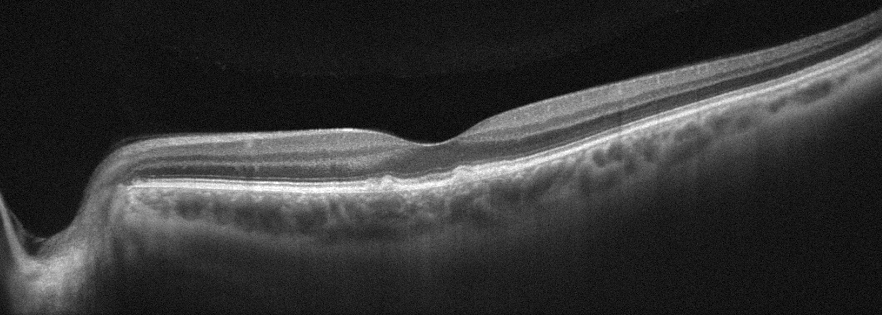 Oculus sinister. Optical coherence tomography B-scan.
Impression: age-related macular degeneration.